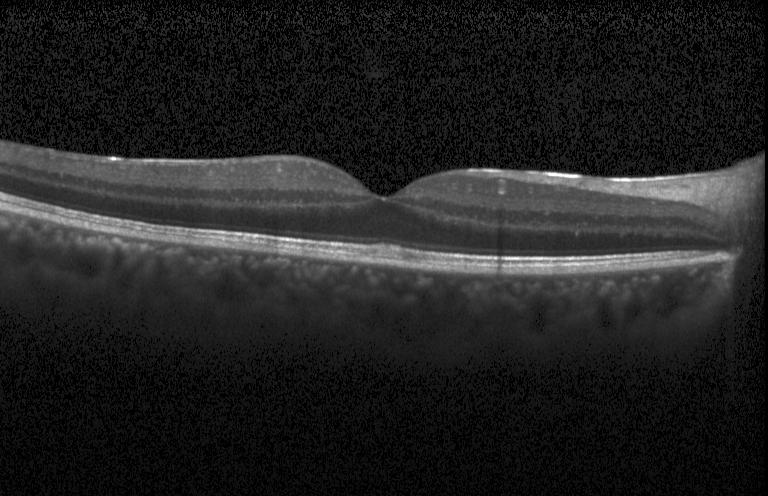

Spectral-domain OCT, centered on the fovea, OCT B-scan
This B-scan demonstrates neither choroidal neovascularization, diabetic macular edema, nor drusen.